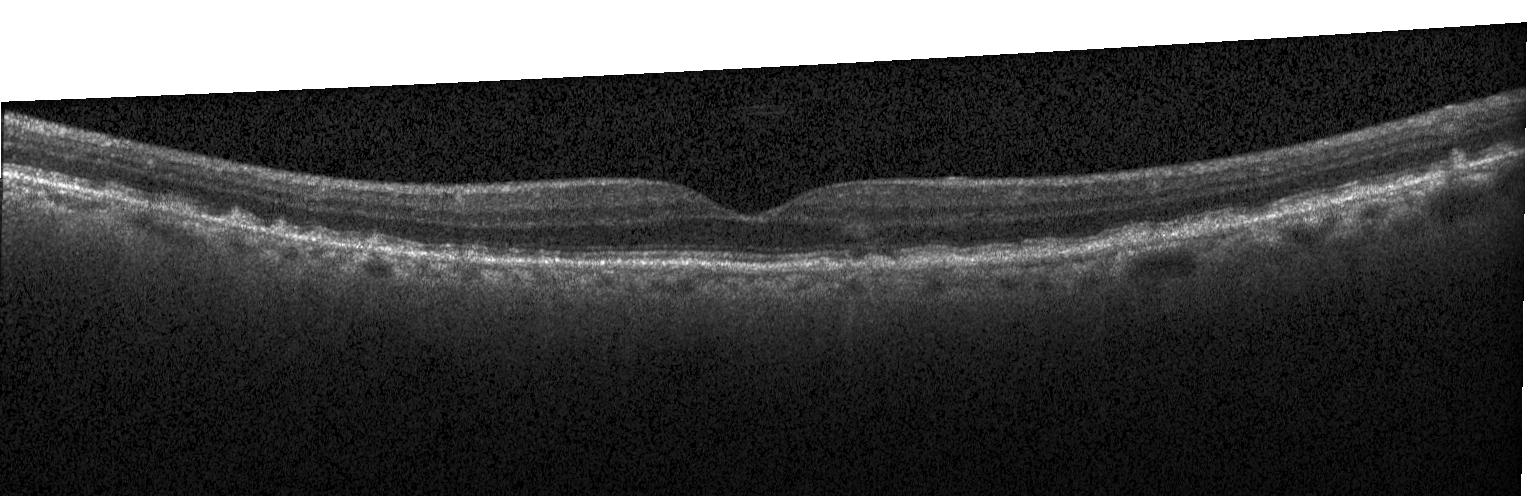
Macular scan. Optical coherence tomography scan — Macular OCT: drusen.